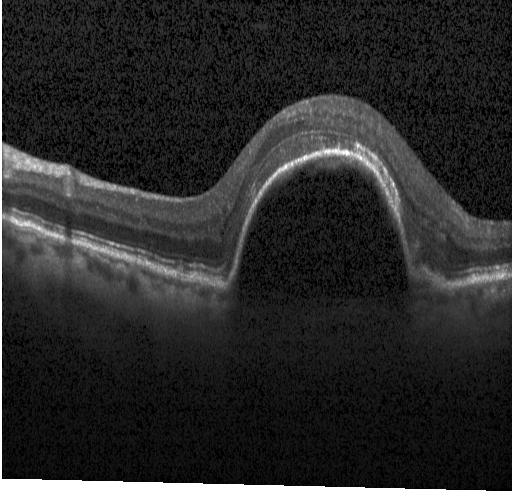 Fovea-centered. Heidelberg Spectralis OCT system. Optical coherence tomography B-scan. Macular OCT: CNV.